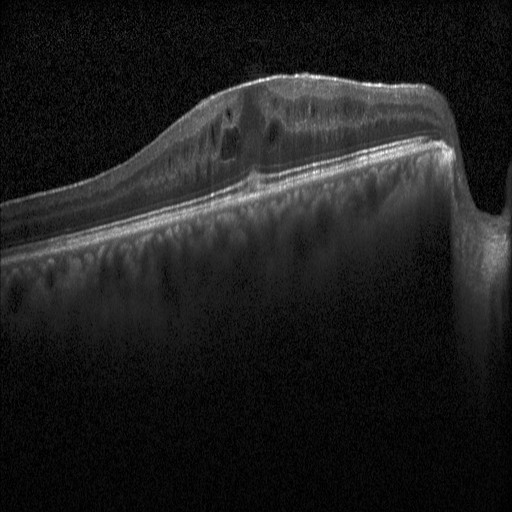 OCT B-scan
The scan shows diabetic macular edema (DME).